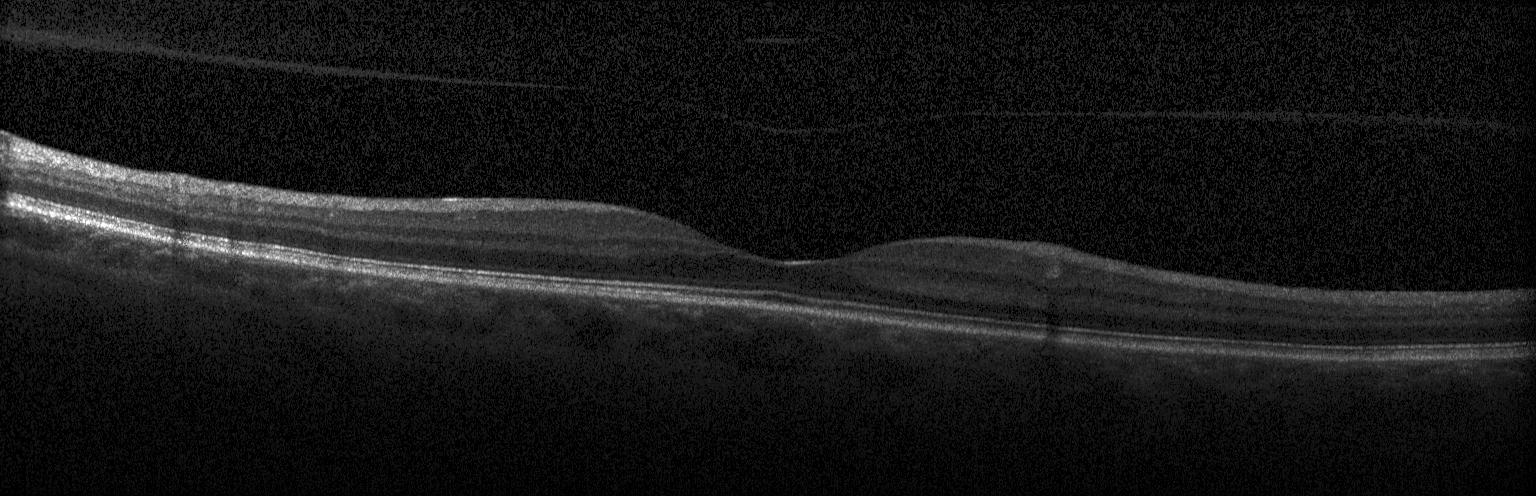

OCT line scan; macular scan.
Impression: neither choroidal neovascularization, diabetic macular edema, nor drusen.